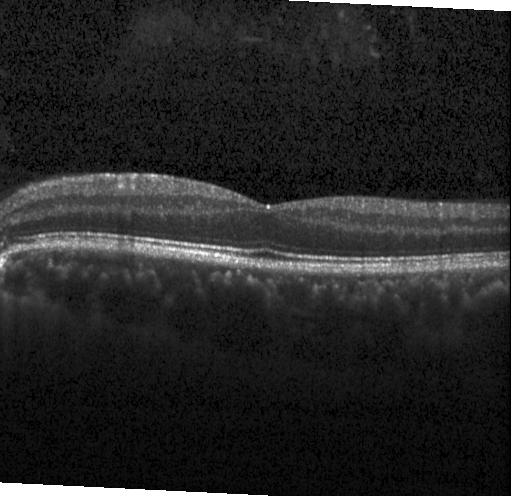

Spectral-domain OCT B-scan: neither CNV, DME, nor drusen.